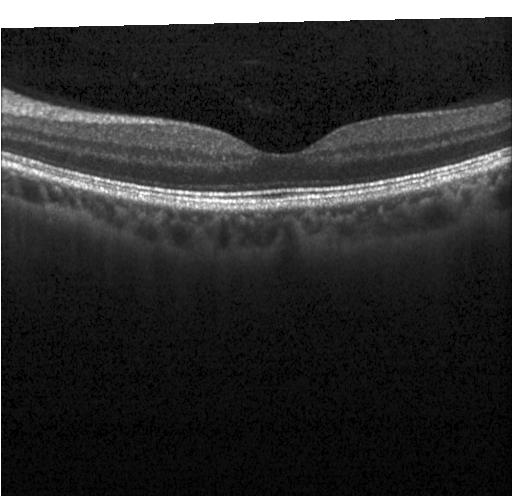
Heidelberg Spectralis; spectral-domain optical coherence tomography; optical coherence tomography B-scan; through the macula.
Dx: no evidence of choroidal neovascularization, diabetic macular edema, or drusen.